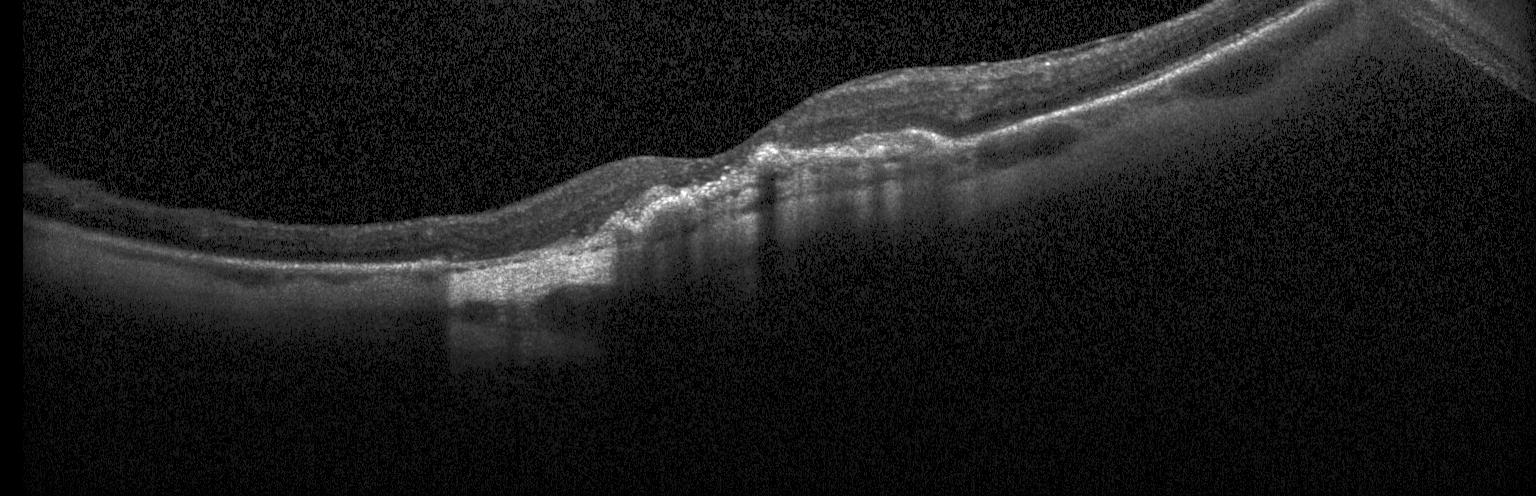 Finding: CNV.